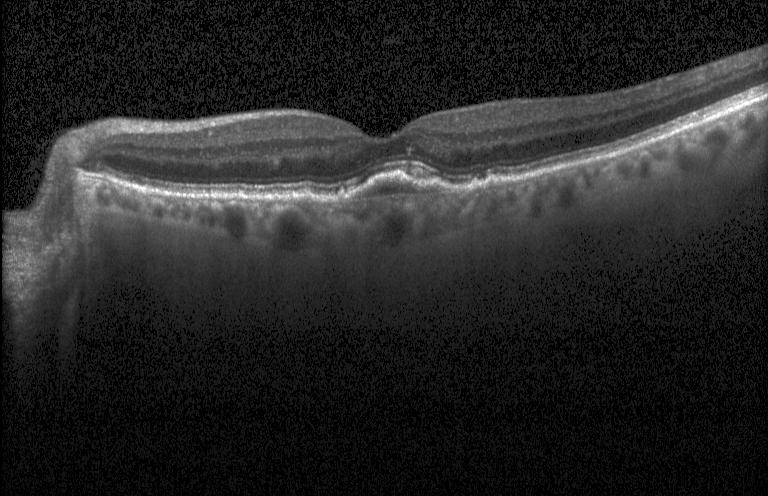 SD-OCT. Instrument: Heidelberg Spectralis. Retinal OCT B-scan. A choroidal neovascular membrane.